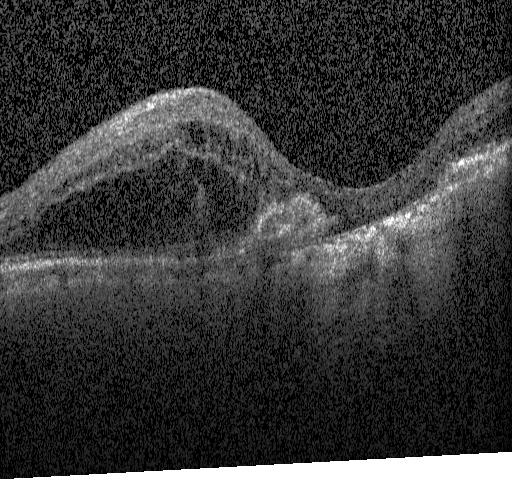

Spectral-domain OCT B-scan: choroidal neovascularization.